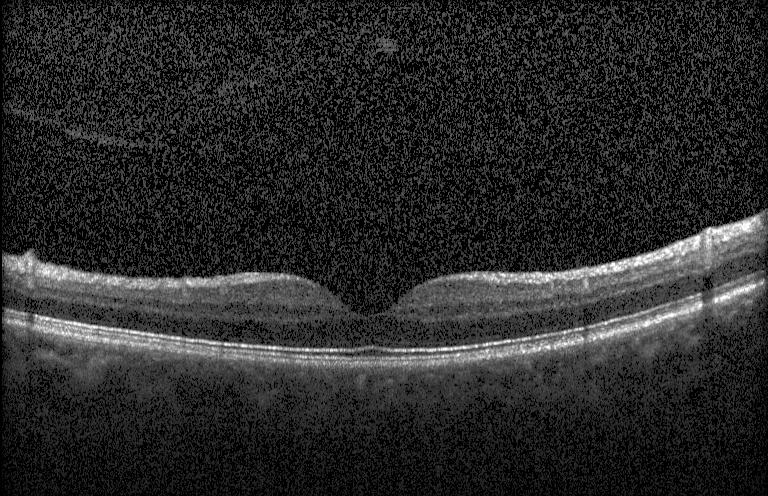

Optical coherence tomography scan · through the macula · instrument: Heidelberg Spectralis · spectral-domain optical coherence tomography — Macular OCT: no evidence of choroidal neovascularization, diabetic macular edema, or drusen.